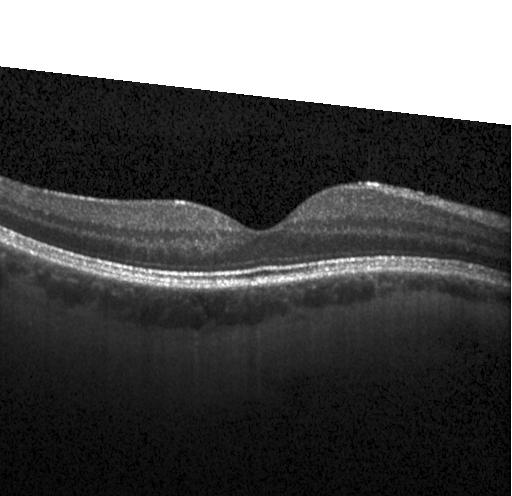

Through the macula, Heidelberg Spectralis OCT system, retinal OCT B-scan
OCT finding: no evidence of choroidal neovascularization, diabetic macular edema, or drusen.